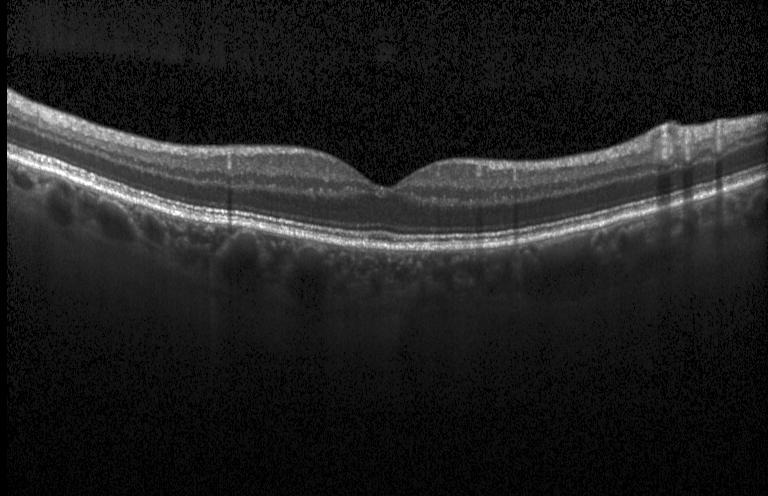
Finding: no choroidal neovascularization, diabetic macular edema, or drusen.